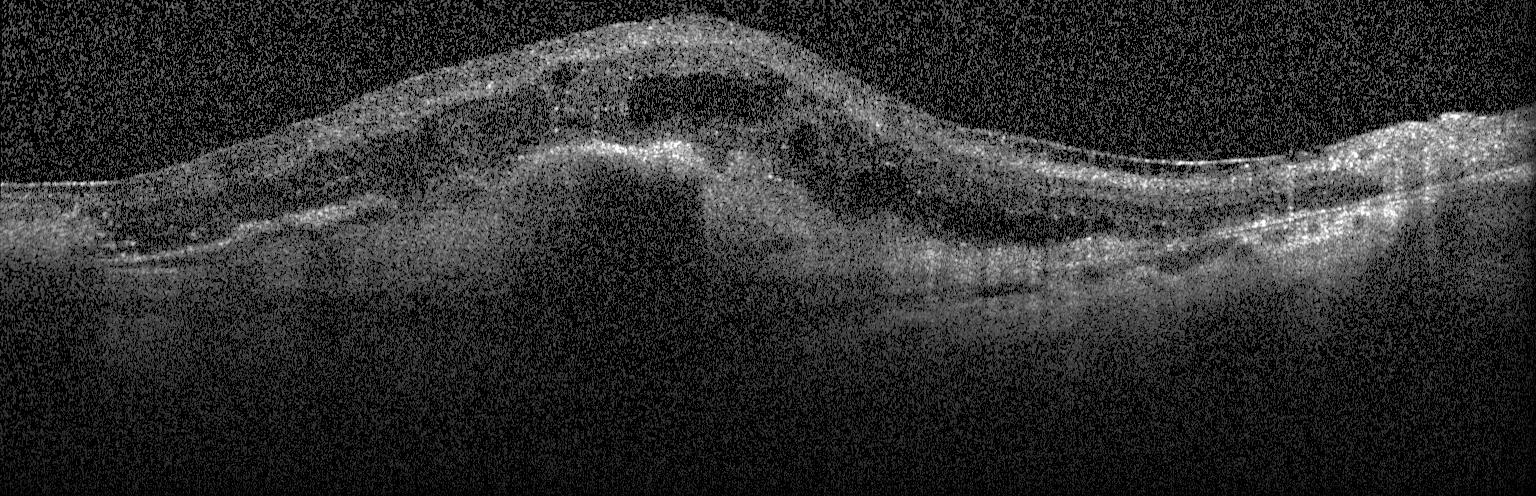
OCT line scan. Spectral-domain optical coherence tomography. Macular scan. Acquired on a Heidelberg Spectralis — Impression: choroidal neovascularization (CNV).